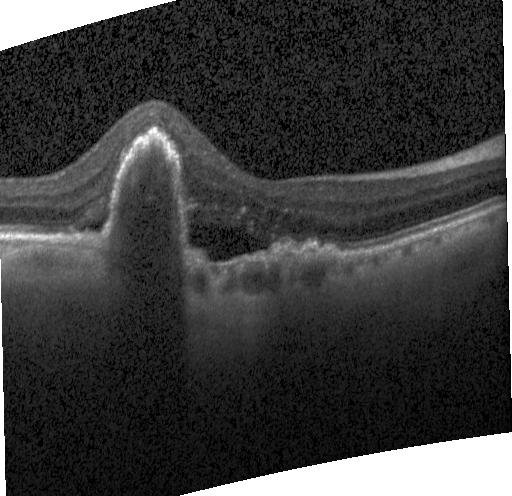
Macular OCT: a choroidal neovascular membrane.